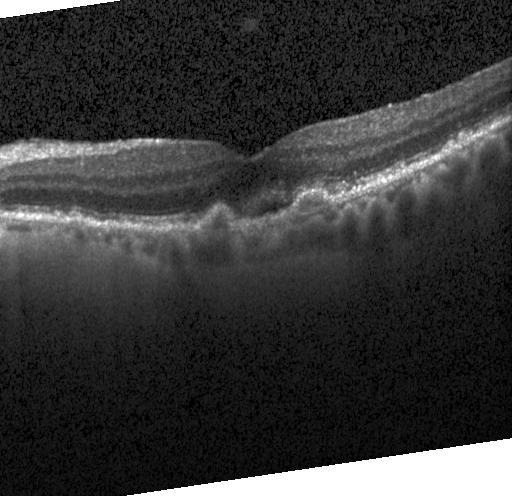
Retinal OCT cross-section — Diagnosis: a choroidal neovascular membrane.